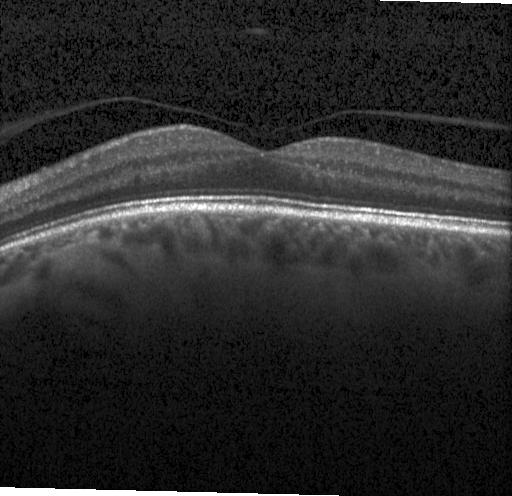
Optical coherence tomography B-scan, through the macula — Dx: no evidence of CNV, DME, or drusen.